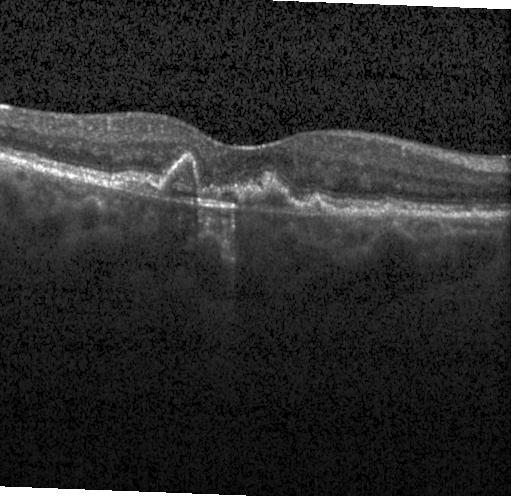
Retinal OCT cross-section showing a choroidal neovascular membrane.